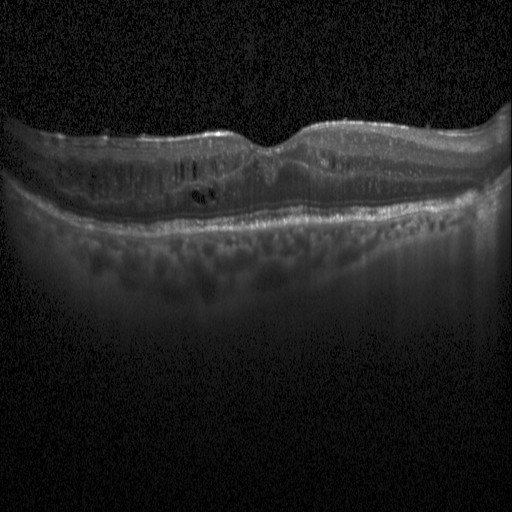 Centered on the fovea; spectral-domain optical coherence tomography; optical coherence tomography B-scan.
The scan shows diabetic macular edema (DME).